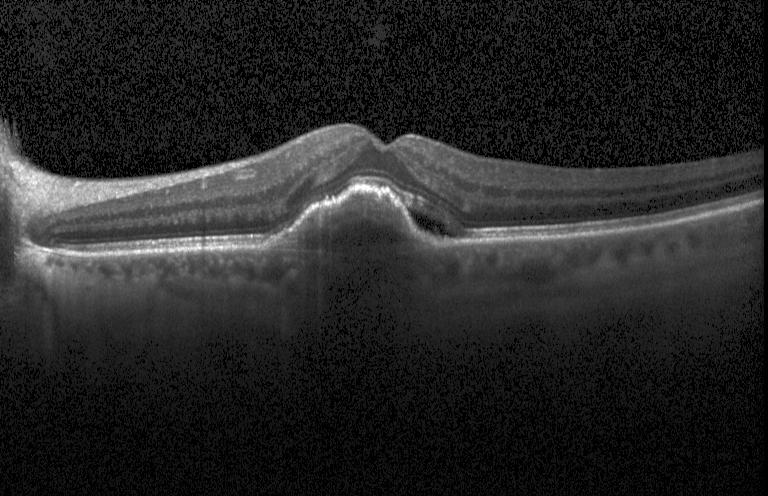
Dx: CNV.